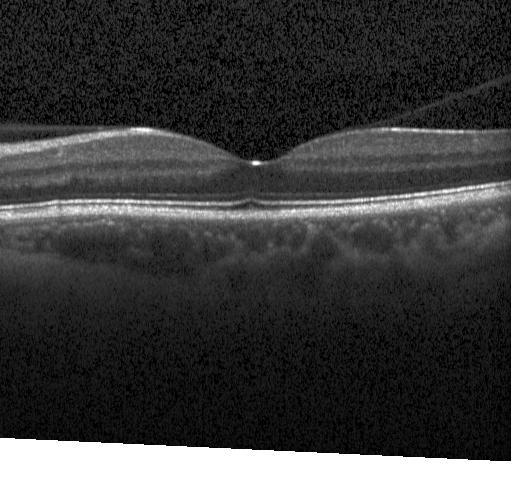 Centered on the fovea · retinal OCT cross-section
The scan shows no evidence of CNV, DME, or drusen.